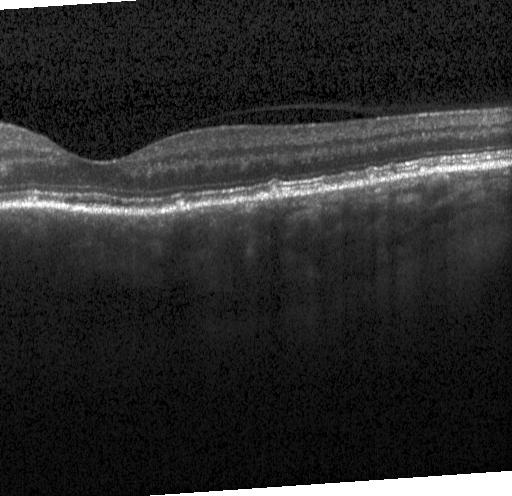 Horizontal scan through the fovea, acquired on a Heidelberg Spectralis, spectral-domain optical coherence tomography, OCT line scan.
Finding: multiple drusen.